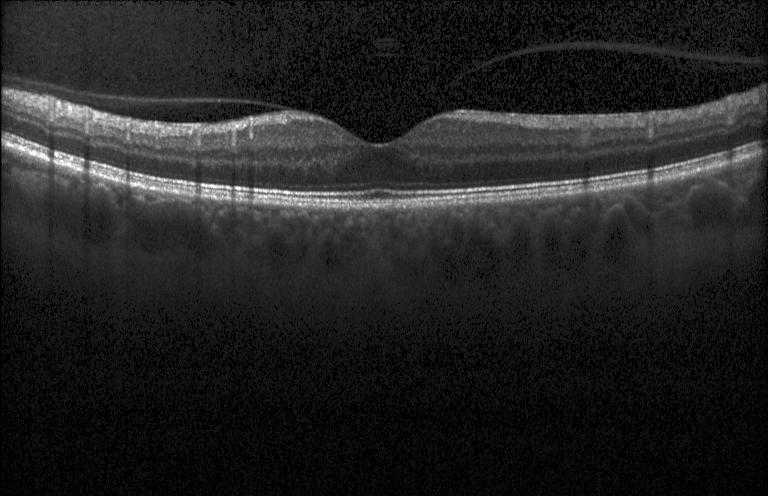 Instrument: Heidelberg Spectralis · OCT B-scan · macular scan.
OCT finding: no CNV, no DME, and no drusen.